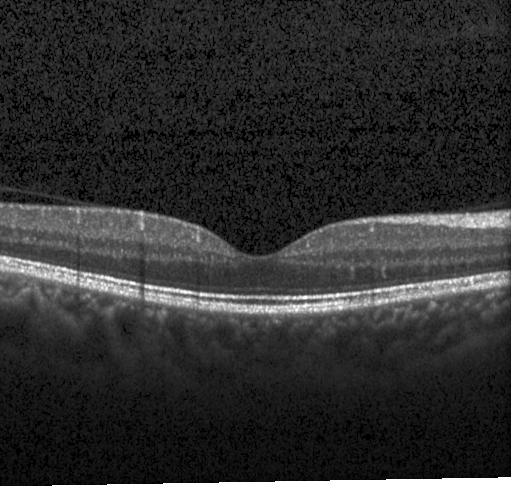

Impression: neither CNV, DME, nor drusen.